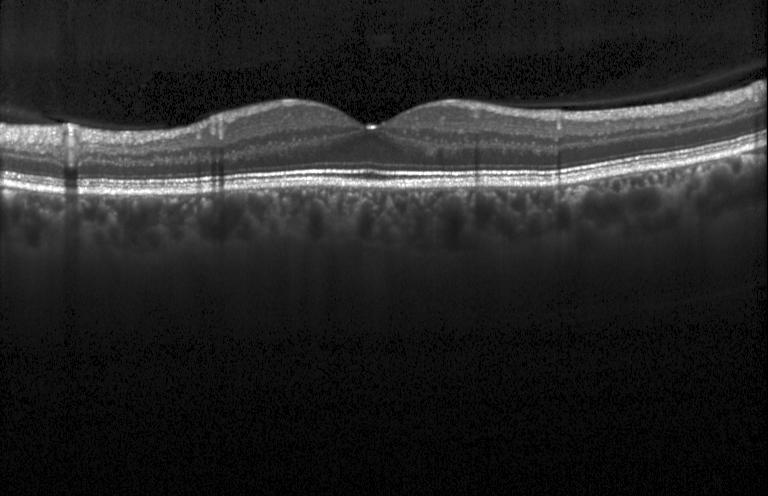 Spectral-domain OCT B-scan: no CNV, no DME, and no drusen.